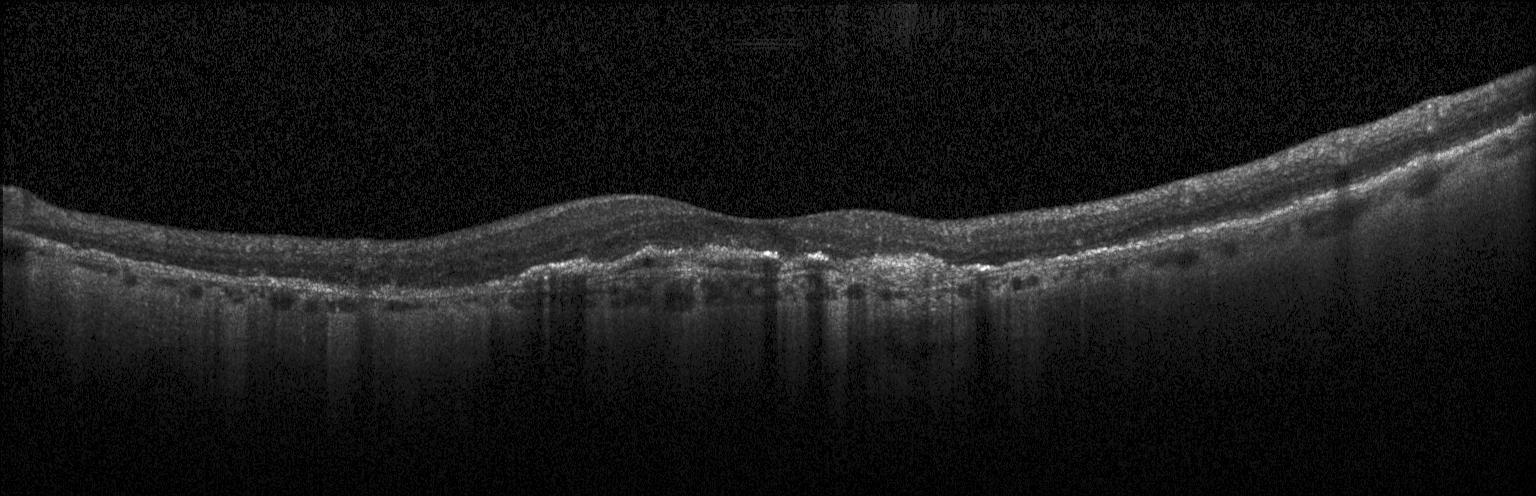
Horizontal scan through the fovea; Heidelberg Spectralis; retinal OCT B-scan. Impression: a choroidal neovascular membrane.